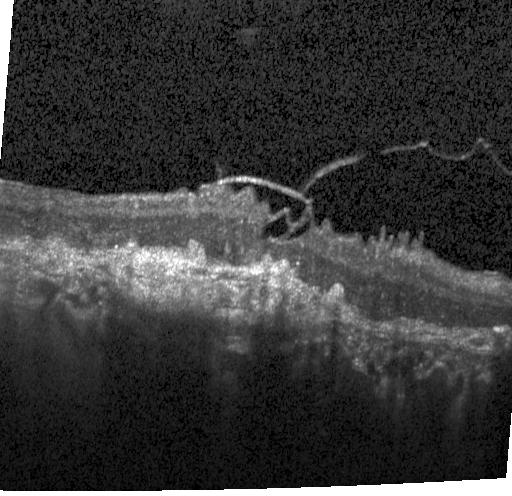

OCT finding: a choroidal neovascular membrane.